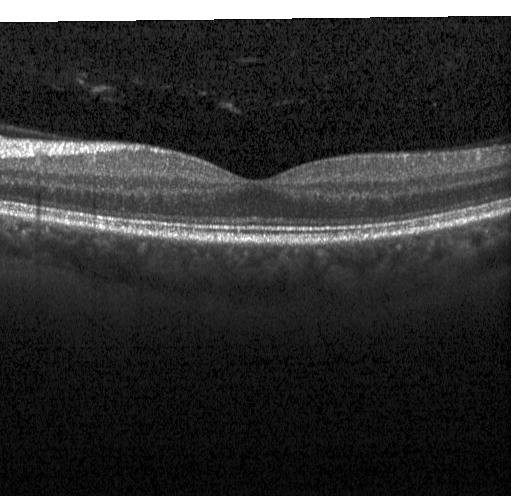

Retinal OCT cross-section showing no choroidal neovascularization, no diabetic macular edema, and no drusen.